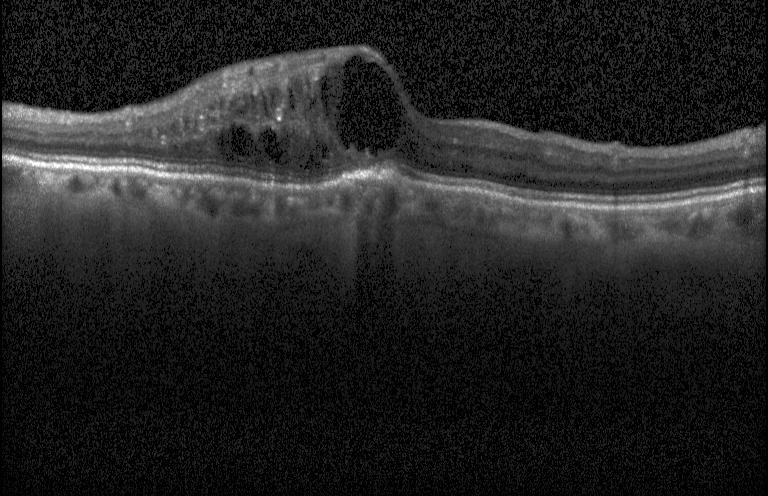

Horizontal scan through the fovea. Retinal OCT cross-section. Spectral-domain optical coherence tomography. The scan shows DME.